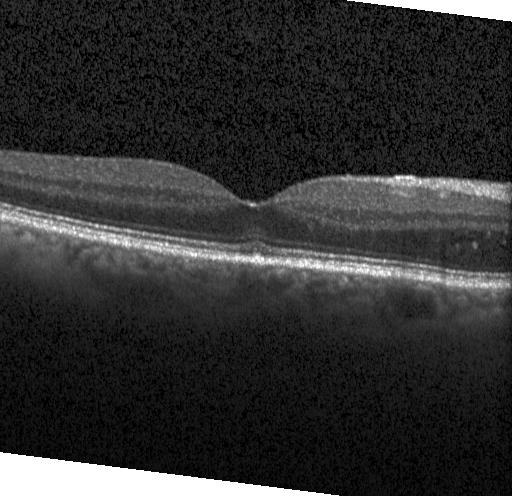 Spectral-domain OCT B-scan: no CNV, DME, or drusen.